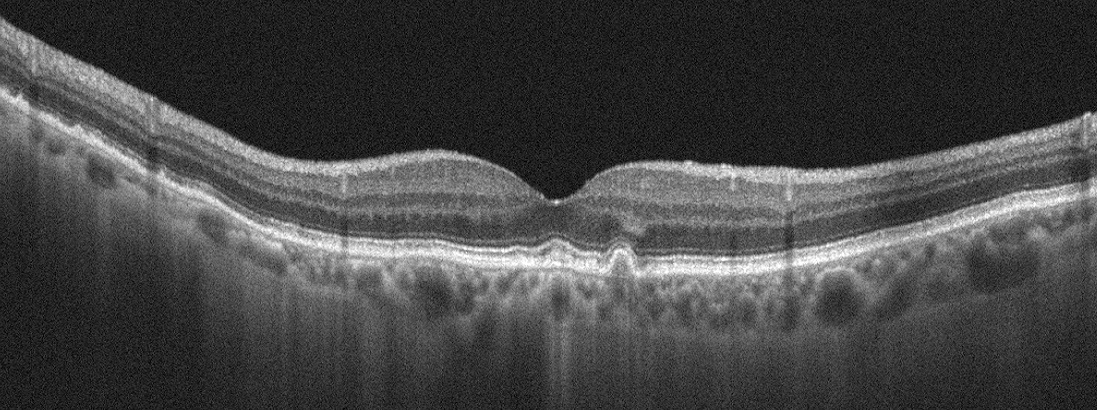 Optical coherence tomography B-scan; macular scan; instrument: Optovue Avanti RTVue XR.
This B-scan demonstrates age-related macular degeneration.